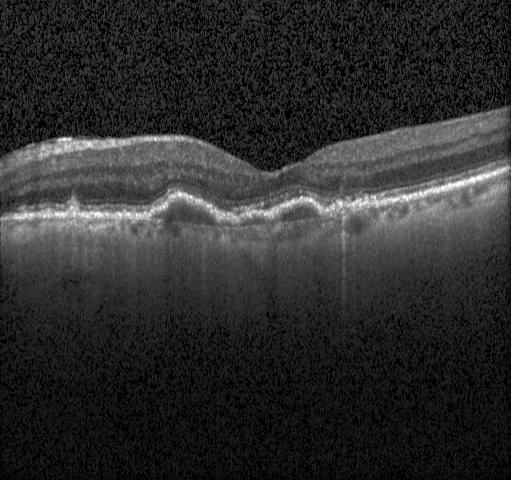

Impression: a choroidal neovascular membrane.